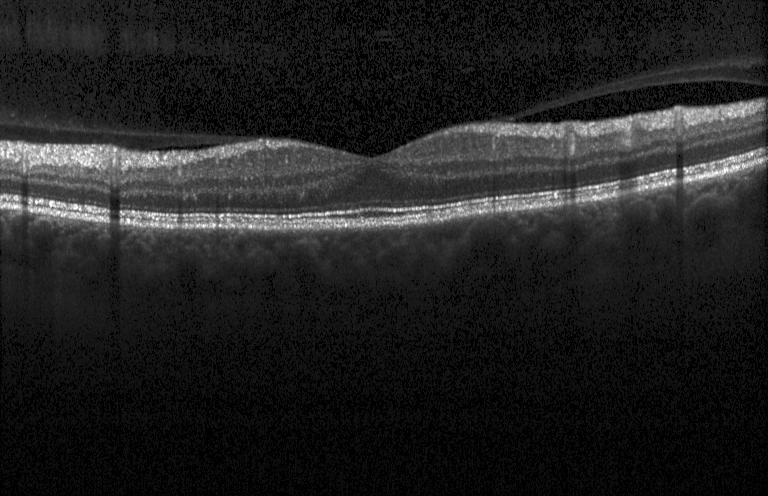
OCT line scan, macular scan.
This B-scan demonstrates neither CNV, DME, nor drusen.